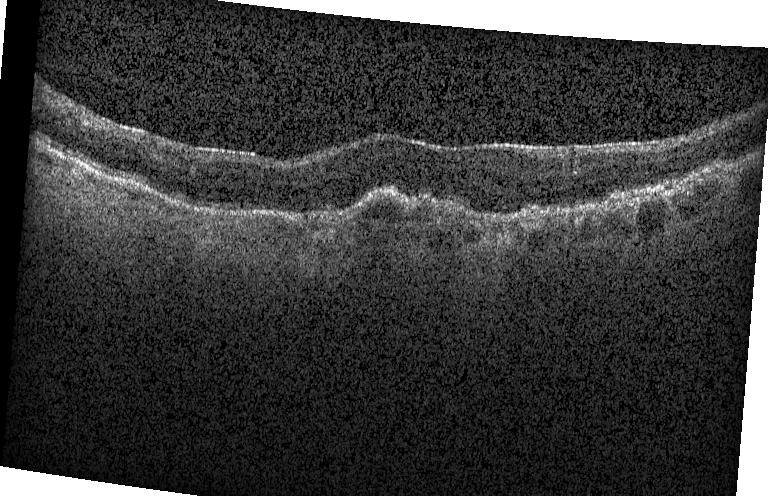 Through the macula; spectral-domain optical coherence tomography; OCT line scan; acquired on a Heidelberg Spectralis — A choroidal neovascular membrane.